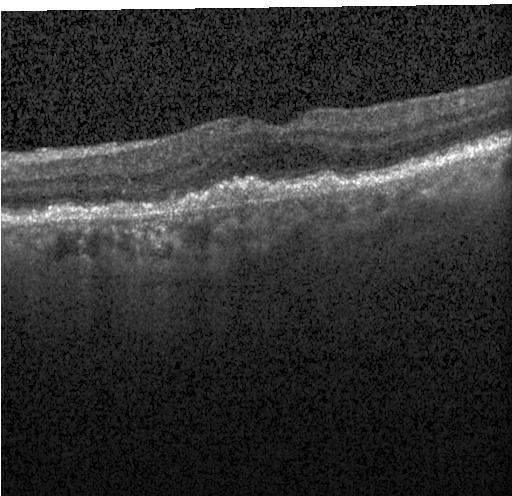
Fovea-centered · spectral-domain optical coherence tomography · OCT B-scan. Finding: a choroidal neovascular membrane.